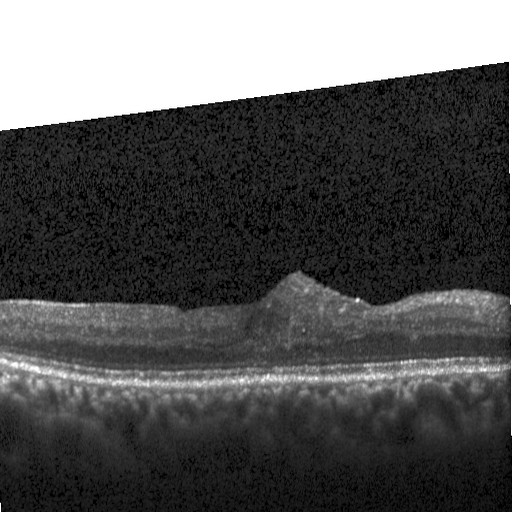
Retinal OCT cross-section showing diabetic macular edema.